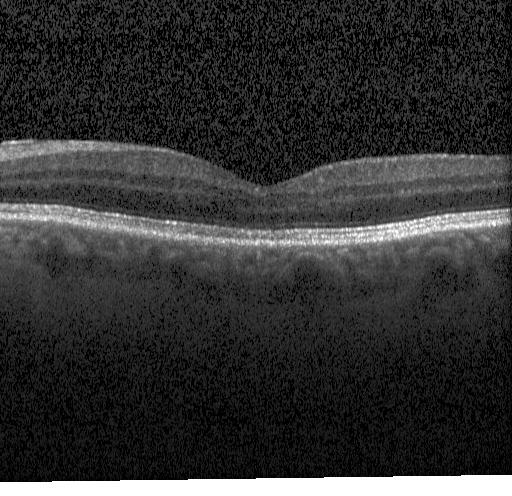
OCT line scan.
This B-scan demonstrates no CNV, no DME, and no drusen.